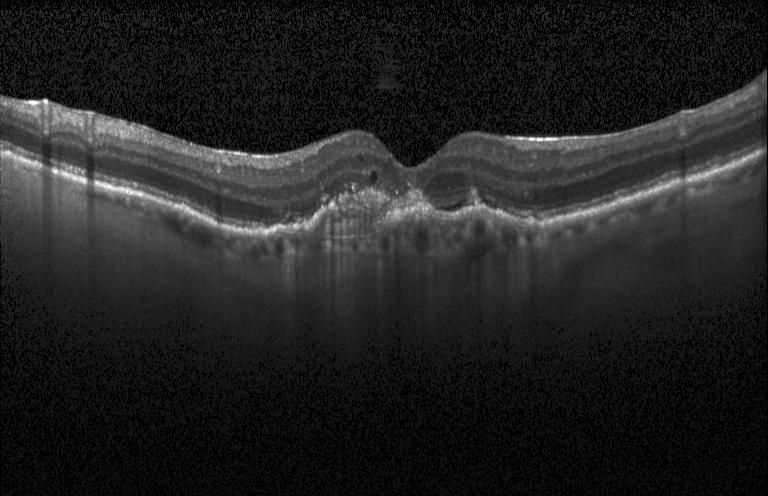 Retinal OCT cross-section showing a choroidal neovascular membrane.